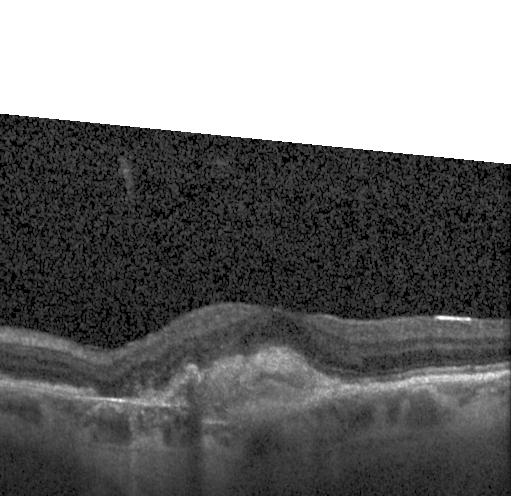 Retinal OCT cross-section showing CNV.